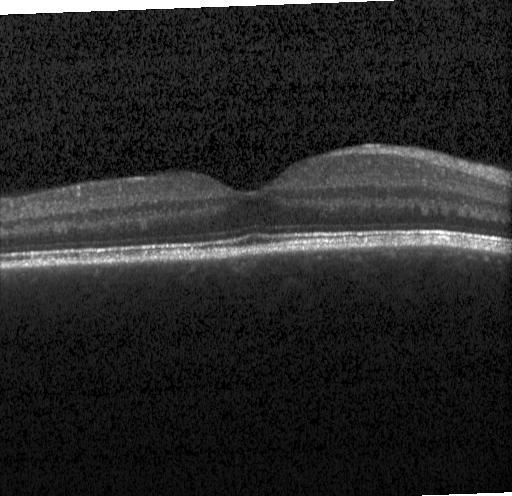
Diagnosis: no evidence of choroidal neovascularization, diabetic macular edema, or drusen.